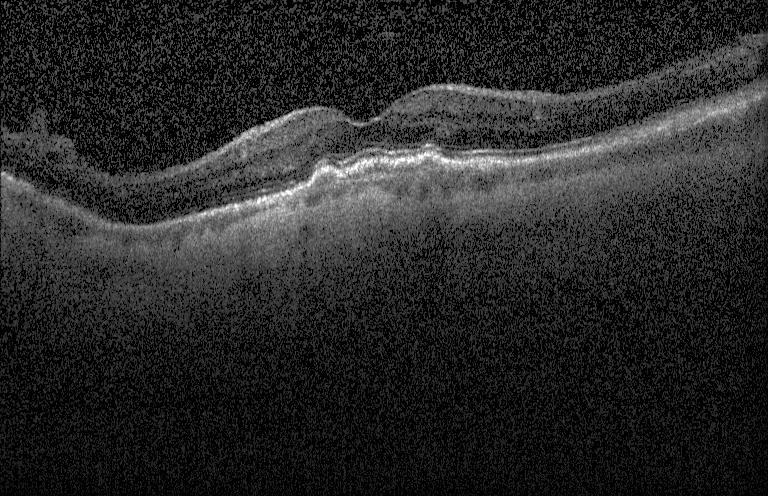
OCT line scan, acquired on a Heidelberg Spectralis, horizontal scan through the fovea, SD-OCT — Macular OCT: a choroidal neovascular membrane.